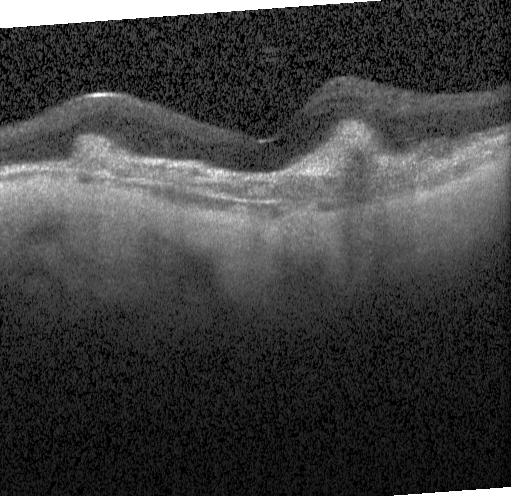

Through the macula · retinal OCT cross-section.
Diagnosis: a choroidal neovascular membrane.